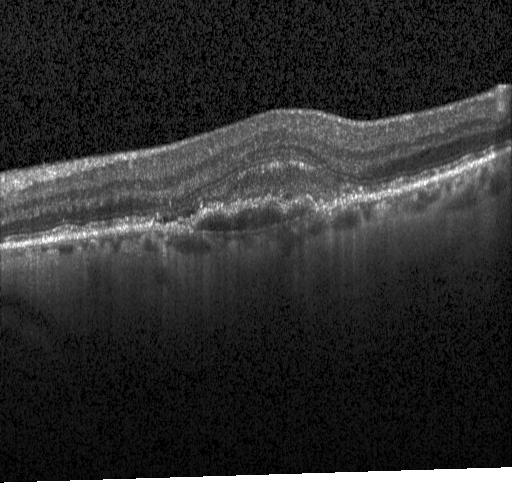

The scan shows CNV.